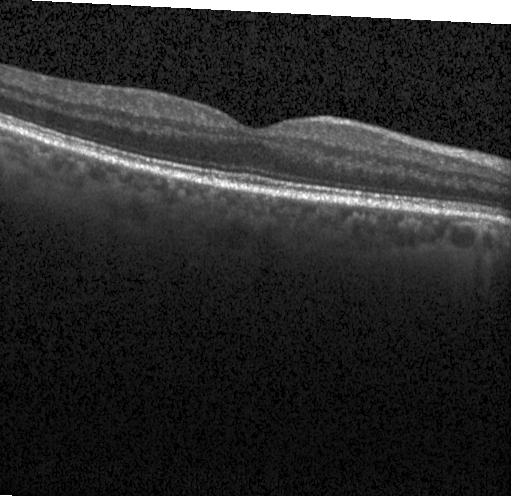 This B-scan demonstrates no choroidal neovascularization, diabetic macular edema, or drusen.